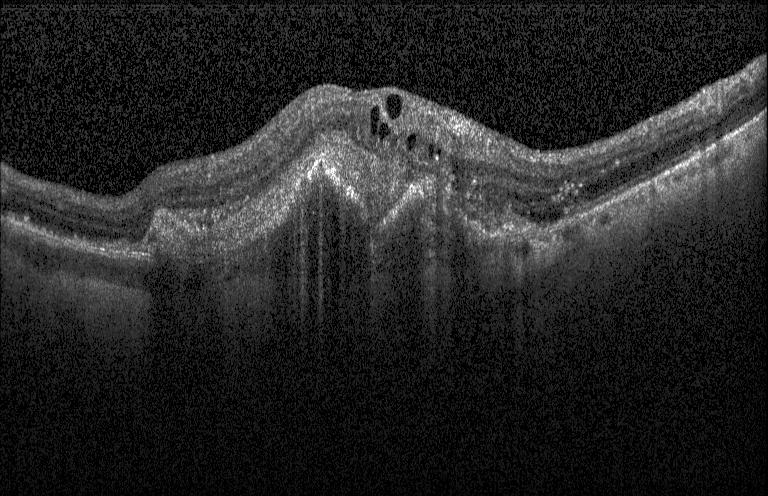
Through the macula · OCT B-scan
Finding: choroidal neovascularization.